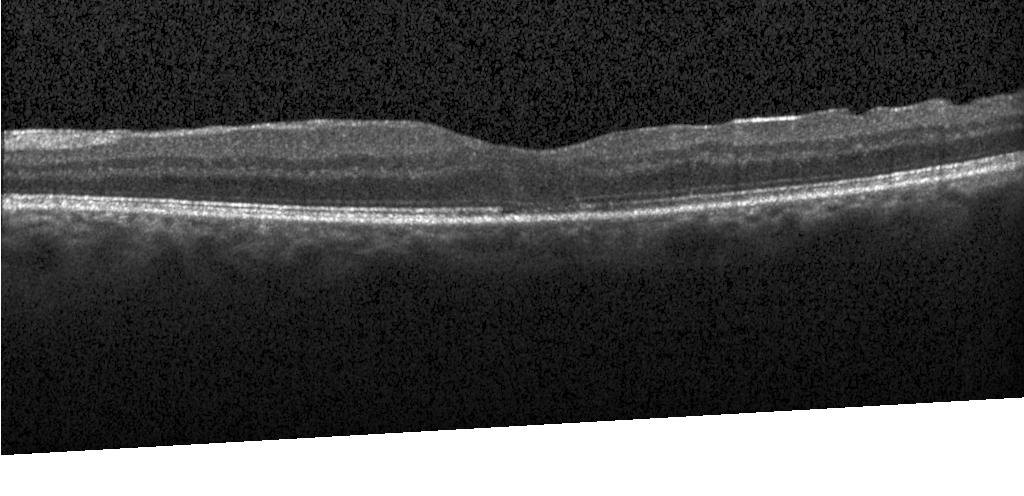

Retinal OCT cross-section. Fovea-centered. Acquired on a Heidelberg Spectralis. Neither choroidal neovascularization, diabetic macular edema, nor drusen.